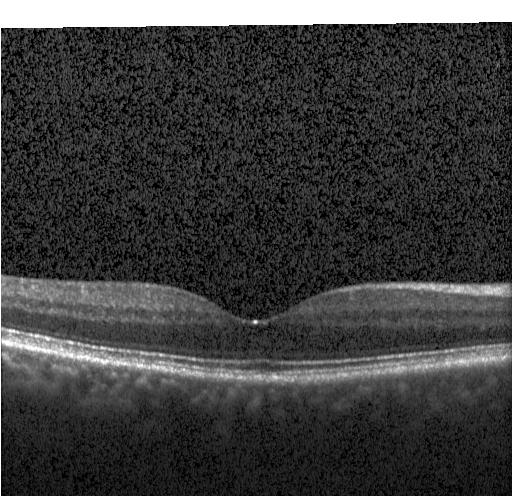 Retinal OCT B-scan; spectral-domain OCT; Heidelberg Spectralis.
Finding: no evidence of choroidal neovascularization, diabetic macular edema, or drusen.